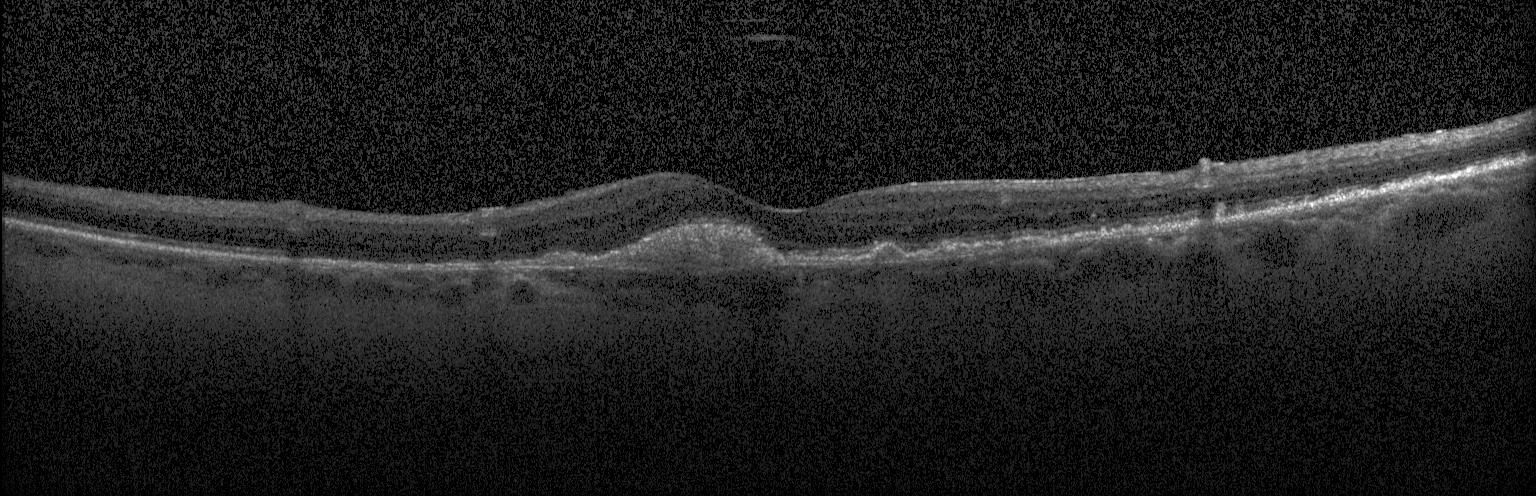
Macular scan. Spectral-domain optical coherence tomography. Retinal OCT B-scan. Heidelberg Spectralis
CNV.